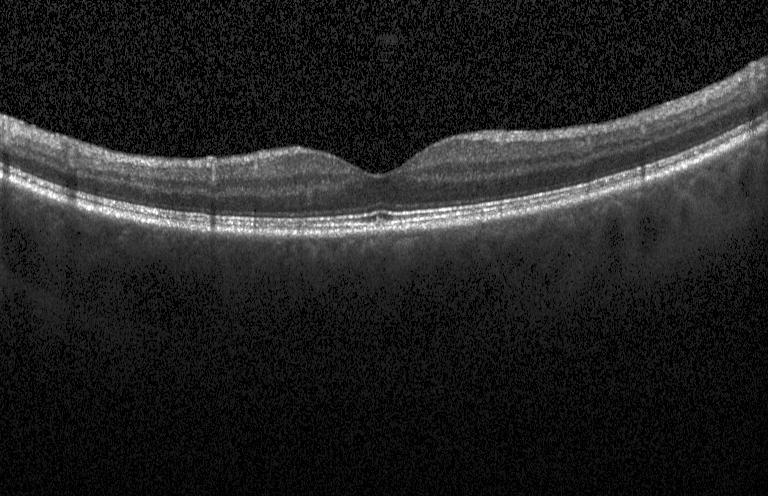
Instrument: Heidelberg Spectralis, spectral-domain optical coherence tomography, horizontal scan through the fovea, retinal OCT B-scan
Dx: no CNV, no DME, and no drusen.